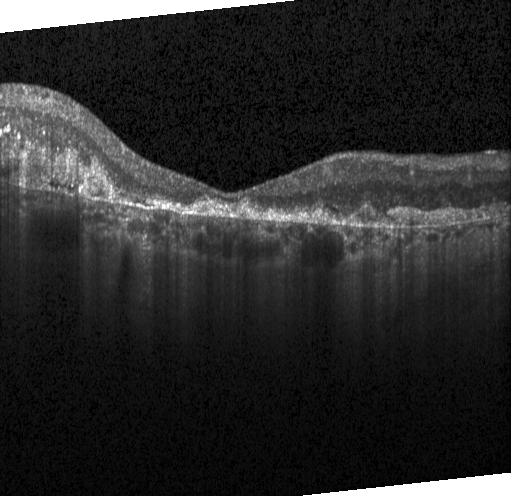
Heidelberg Spectralis OCT system. OCT B-scan. Spectral-domain optical coherence tomography. Centered on the fovea
Finding: a choroidal neovascular membrane.